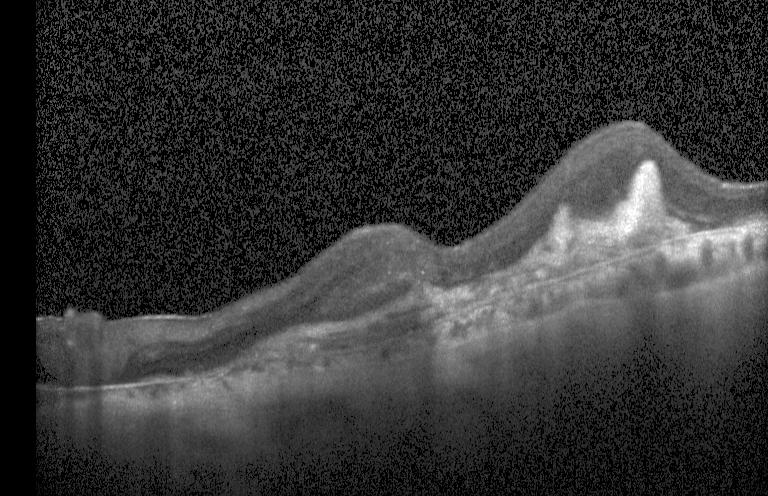

SD-OCT; horizontal scan through the fovea; retinal OCT B-scan — Impression: choroidal neovascularization.